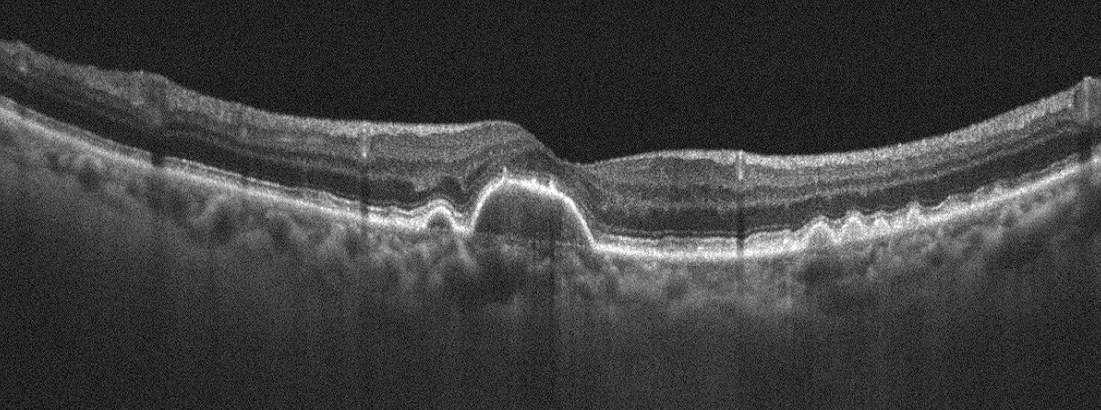
Optical coherence tomography scan. Finding: AMD.